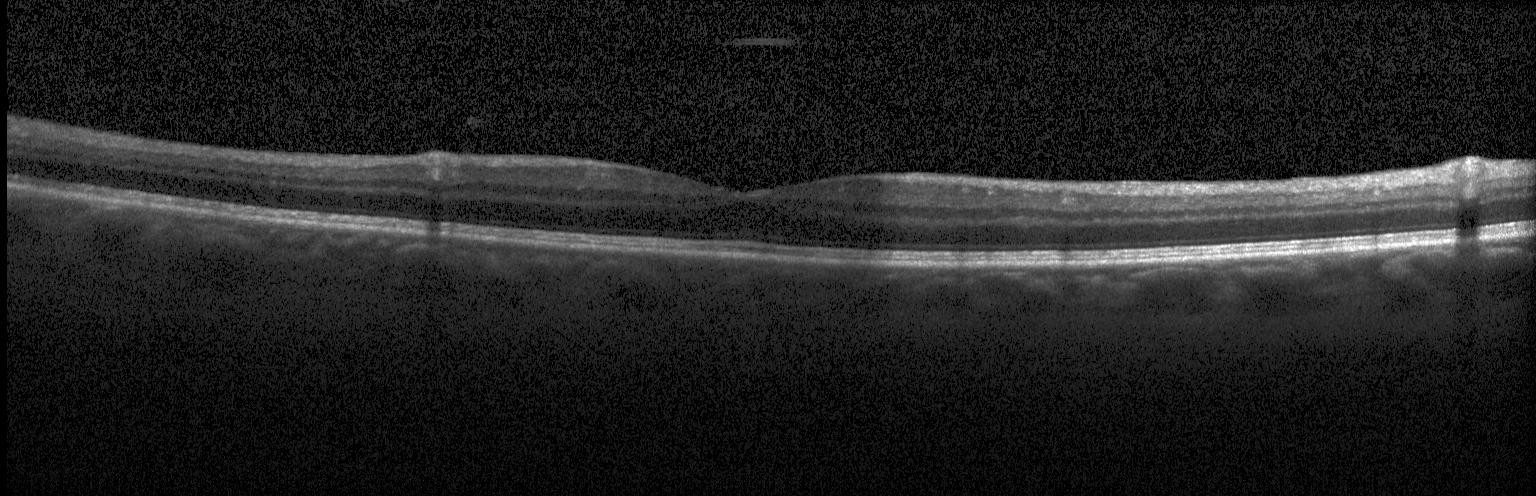
Dx: no evidence of CNV, DME, or drusen.